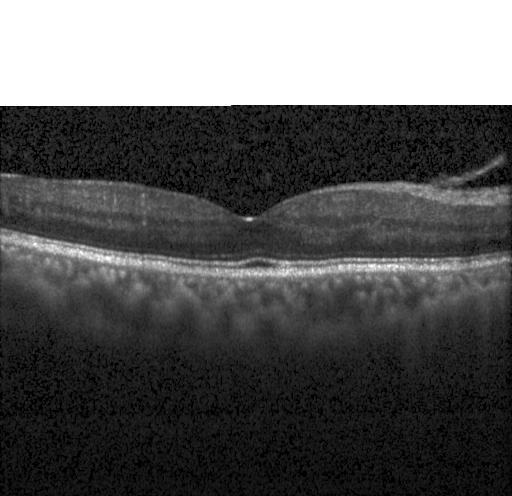
Through the macula. OCT B-scan — OCT finding: neither choroidal neovascularization, diabetic macular edema, nor drusen.